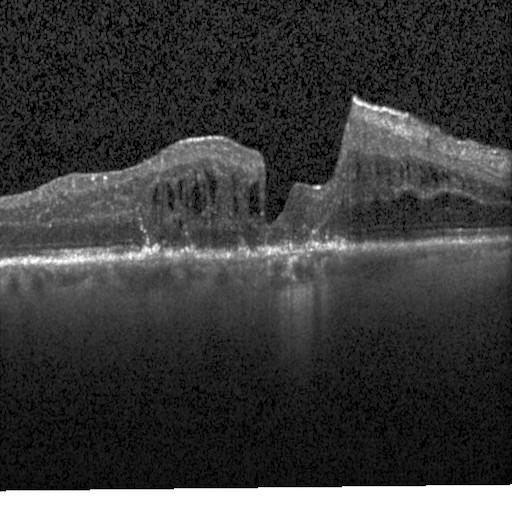 Optical coherence tomography scan.
Dx: diabetic macular edema (DME).